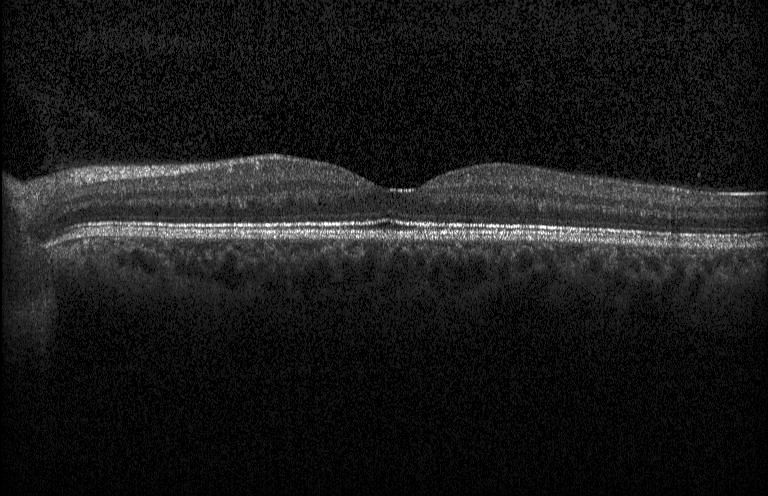
Diagnosis: neither choroidal neovascularization, diabetic macular edema, nor drusen.